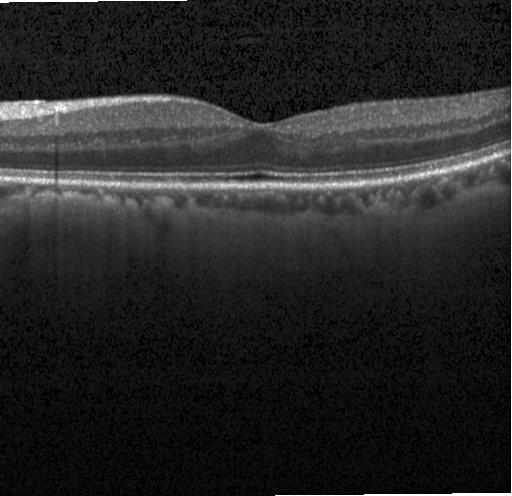

Impression: neither CNV, DME, nor drusen.